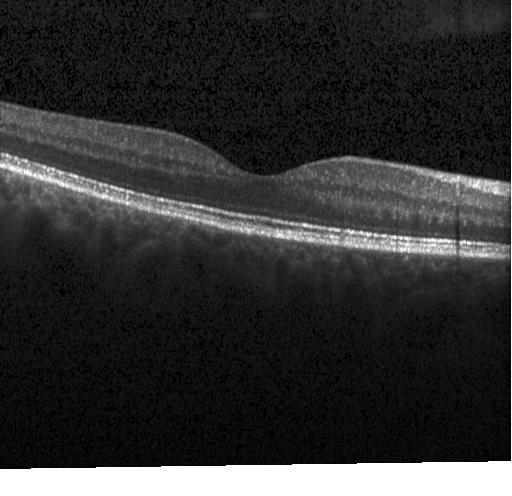 Macular OCT: neither choroidal neovascularization, diabetic macular edema, nor drusen.